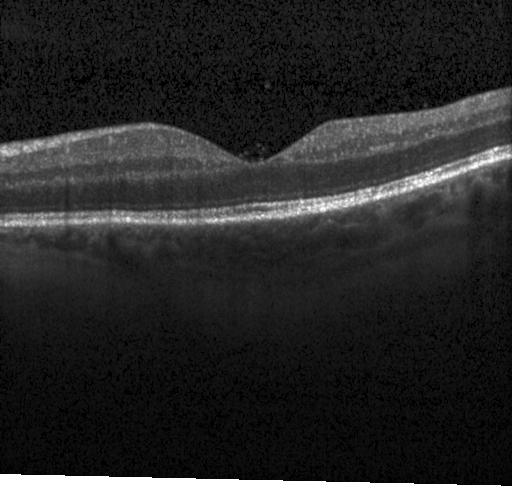 Neither choroidal neovascularization, diabetic macular edema, nor drusen.